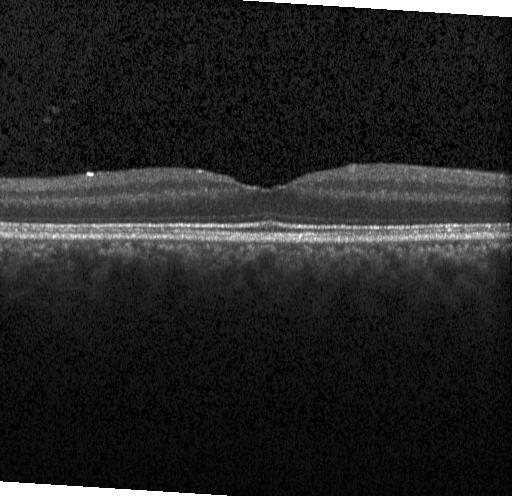
OCT B-scan.
Impression: no choroidal neovascularization, diabetic macular edema, or drusen.